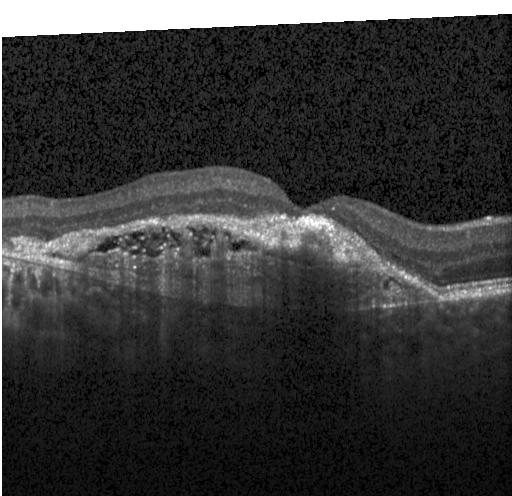

OCT B-scan.
A choroidal neovascular membrane.